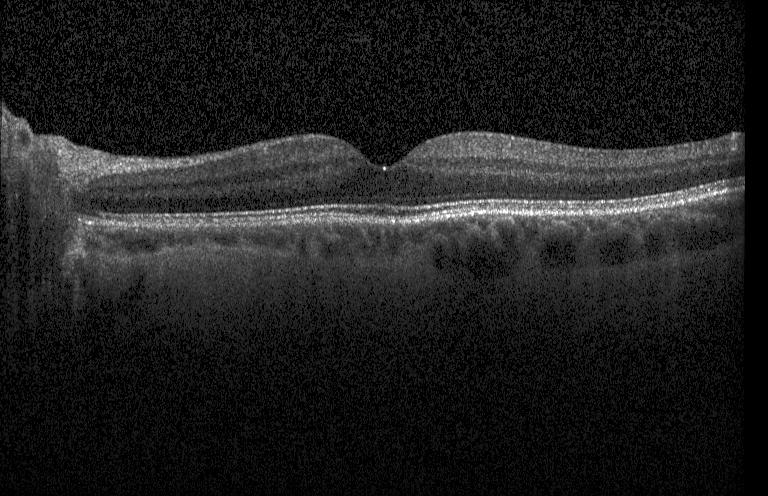 Retinal OCT cross-section. Centered on the fovea. Heidelberg Spectralis. SD-OCT.
Macular OCT: no CNV, DME, or drusen.